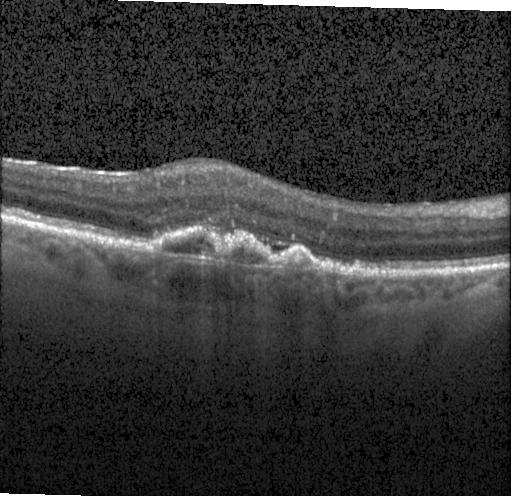
Horizontal scan through the fovea. Optical coherence tomography scan. Heidelberg Spectralis. Spectral-domain optical coherence tomography — A choroidal neovascular membrane.